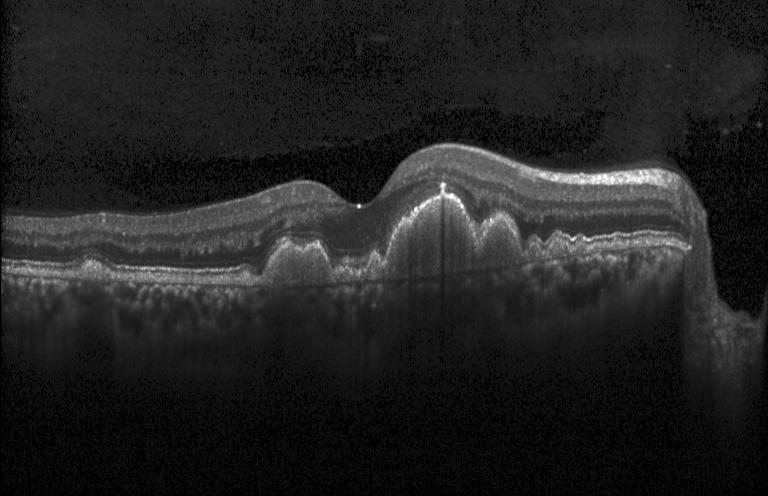

Optical coherence tomography B-scan · macular scan
Diagnosis: multiple drusen.